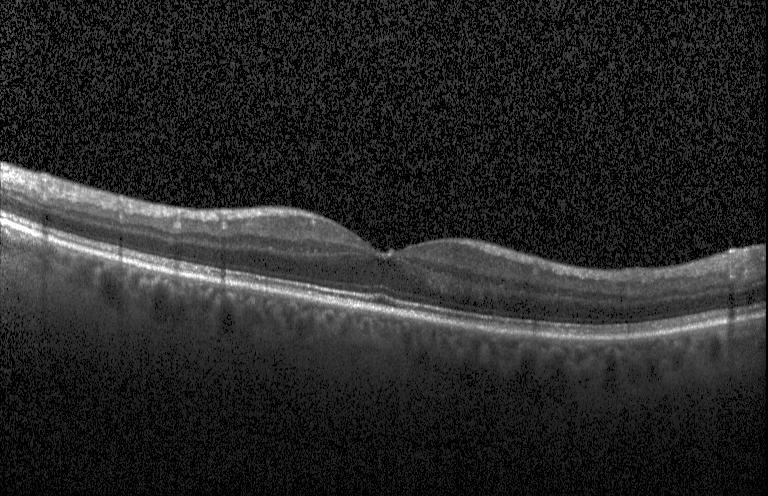 No evidence of choroidal neovascularization, diabetic macular edema, or drusen.